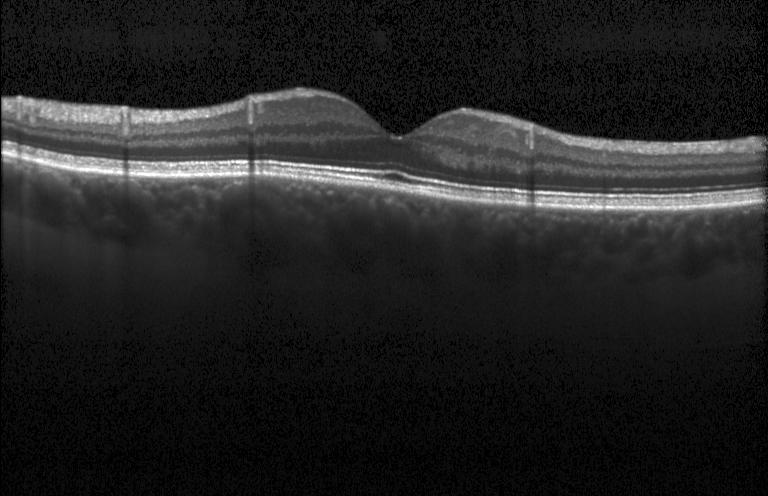
Through the macula. OCT line scan — Finding: neither choroidal neovascularization, diabetic macular edema, nor drusen.